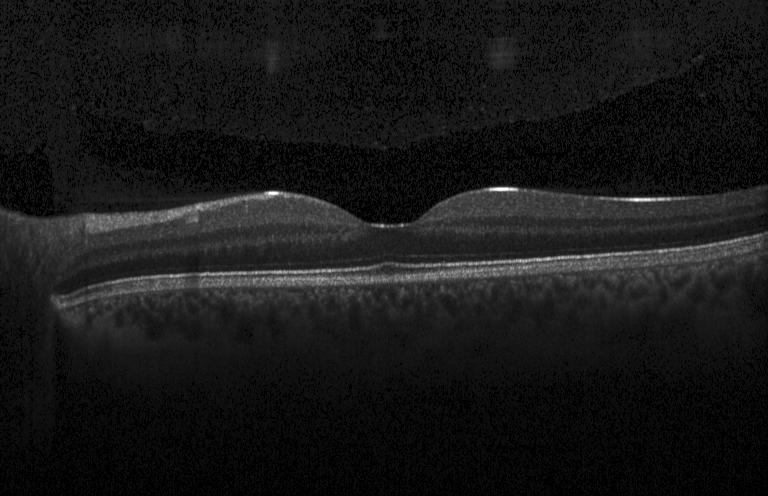
OCT line scan — The scan shows no choroidal neovascularization, no diabetic macular edema, and no drusen.